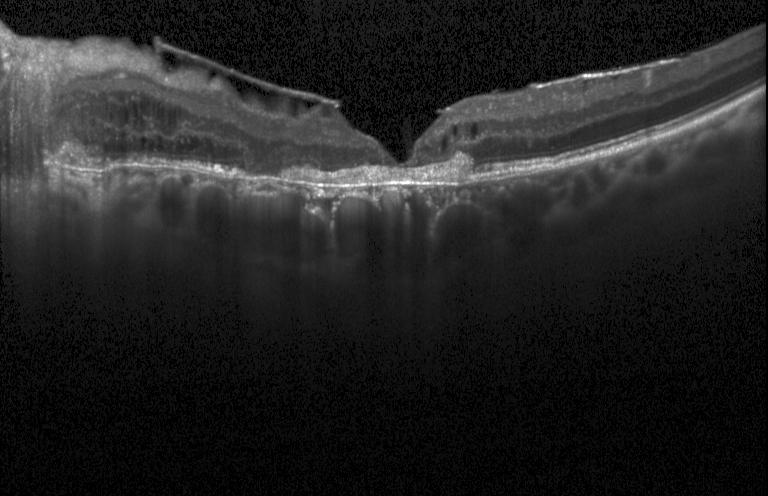

Spectral-domain OCT B-scan: a choroidal neovascular membrane.